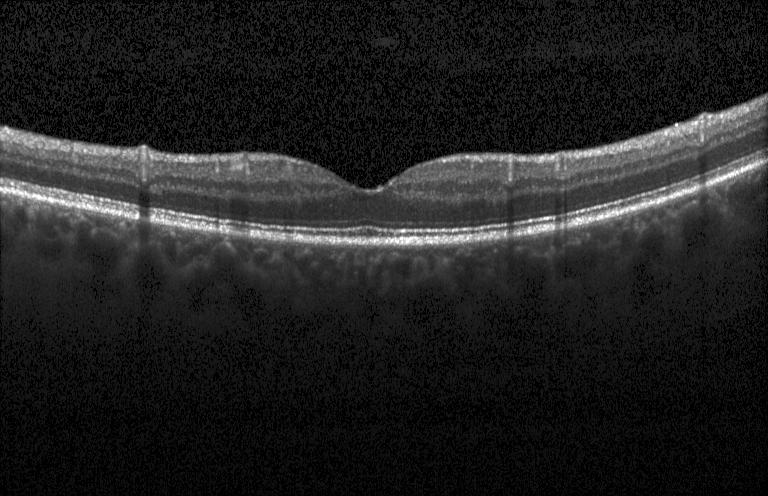
SD-OCT · Heidelberg Spectralis OCT system · through the macula · retinal OCT cross-section. Diagnosis: no choroidal neovascularization, diabetic macular edema, or drusen.